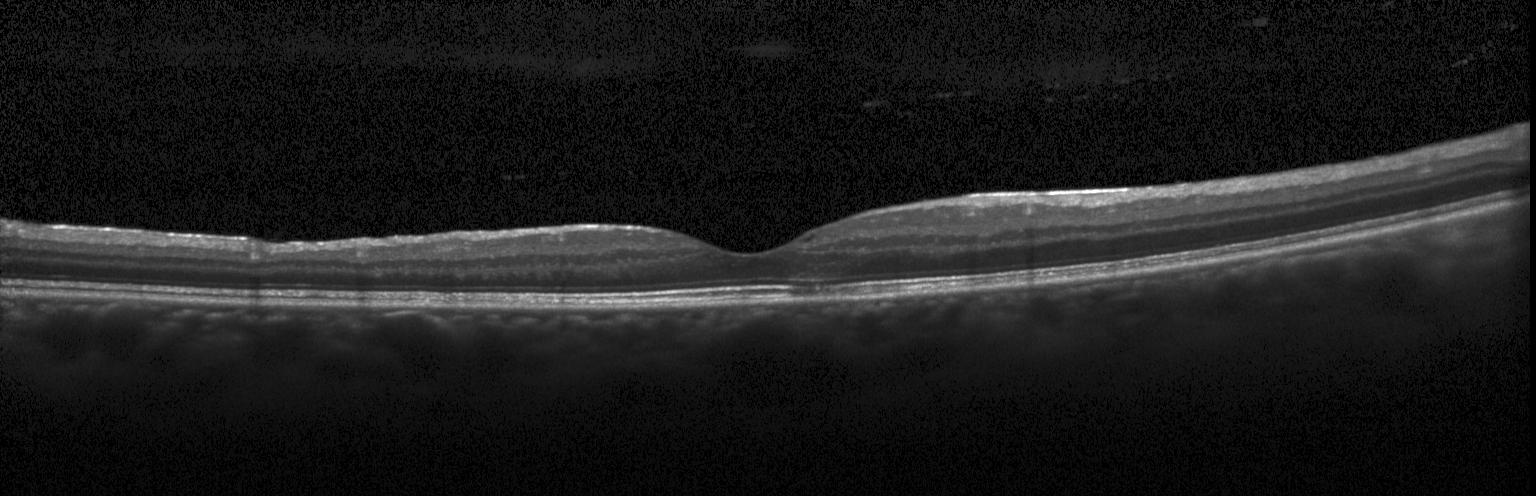 Retinal OCT B-scan.
Finding: no choroidal neovascularization, no diabetic macular edema, and no drusen.